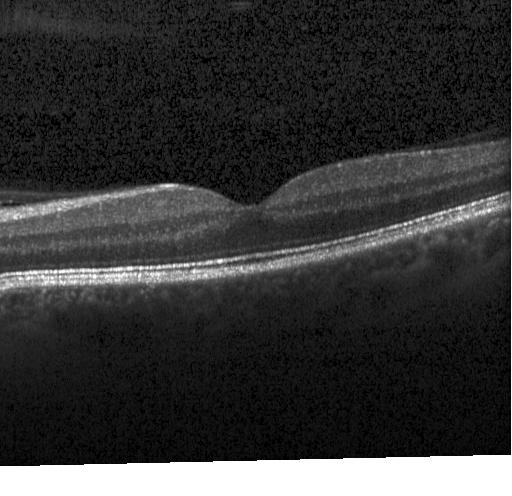

Through the macula, instrument: Heidelberg Spectralis, OCT line scan, SD-OCT.
The scan shows no evidence of choroidal neovascularization, diabetic macular edema, or drusen.